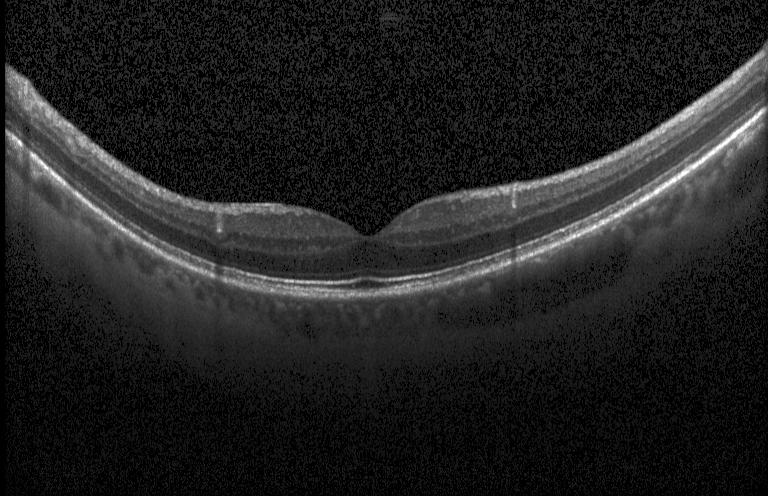 Impression: no CNV, DME, or drusen.